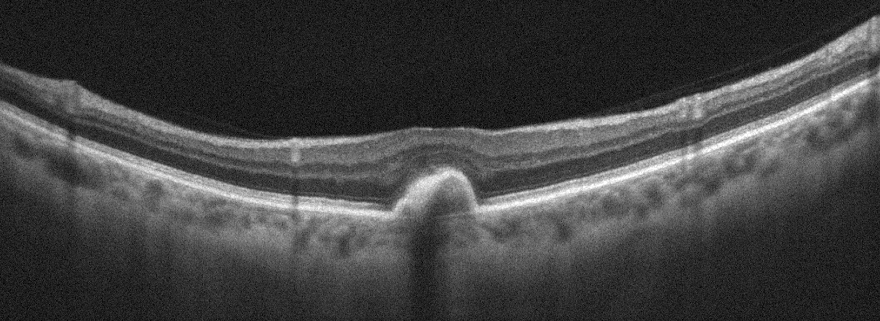

Retinal OCT B-scan; OS. Diagnosis: age-related macular degeneration.